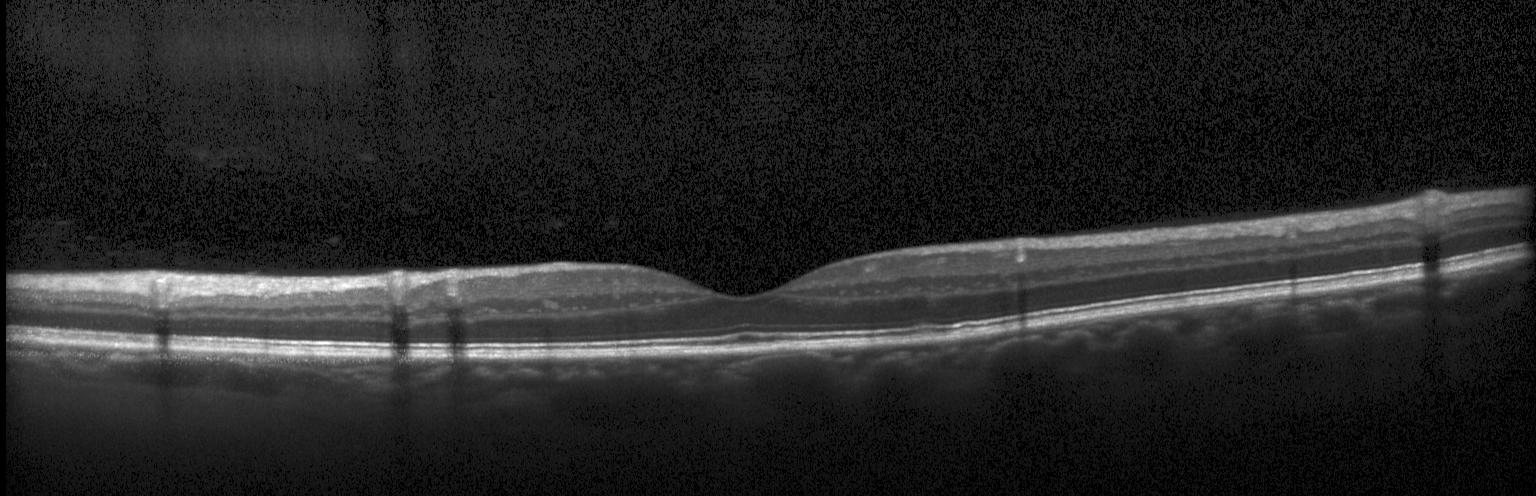 OCT finding: no evidence of choroidal neovascularization, diabetic macular edema, or drusen.